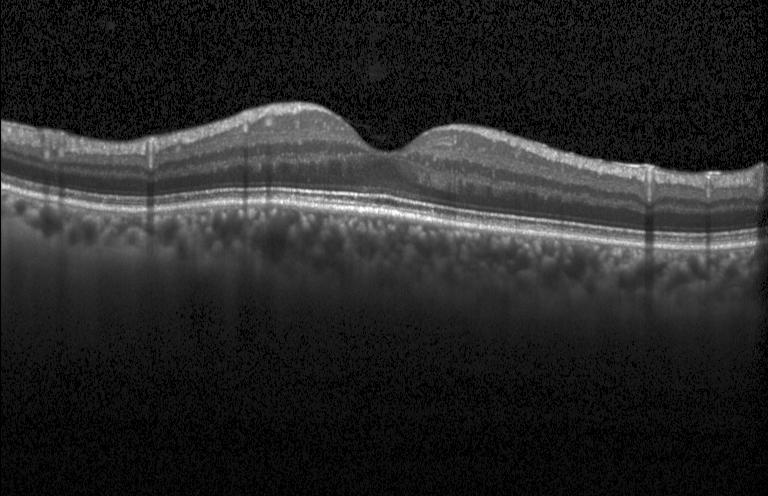
Spectral-domain OCT. Heidelberg Spectralis. OCT line scan. Horizontal scan through the fovea
Diagnosis: no choroidal neovascularization, no diabetic macular edema, and no drusen.